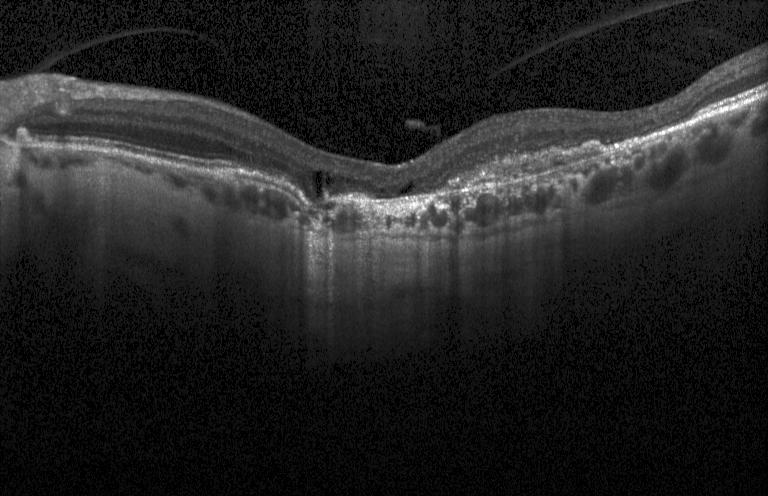

SD-OCT, retinal OCT cross-section, Heidelberg Spectralis OCT system, macular scan.
Dx: a choroidal neovascular membrane.